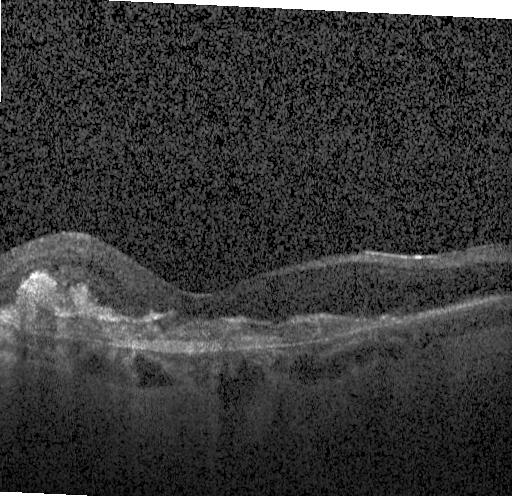

Optical coherence tomography B-scan. Macular scan. Heidelberg Spectralis OCT system. Spectral-domain optical coherence tomography.
Assessment: a choroidal neovascular membrane.